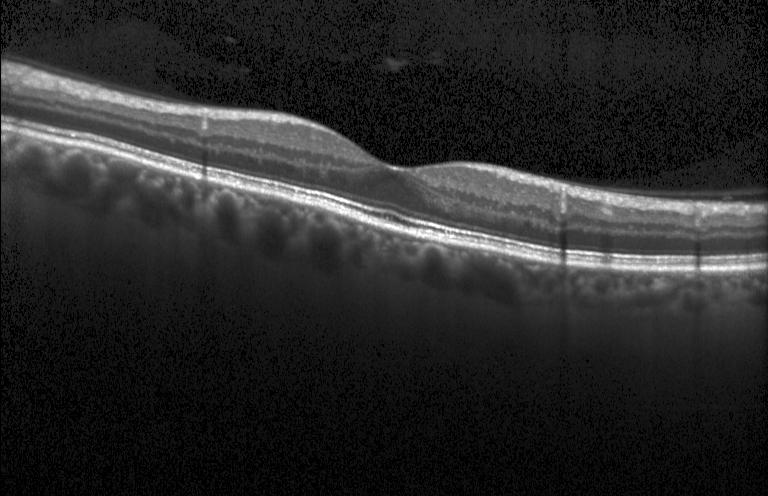
Horizontal scan through the fovea; OCT B-scan.
Impression: no choroidal neovascularization, no diabetic macular edema, and no drusen.